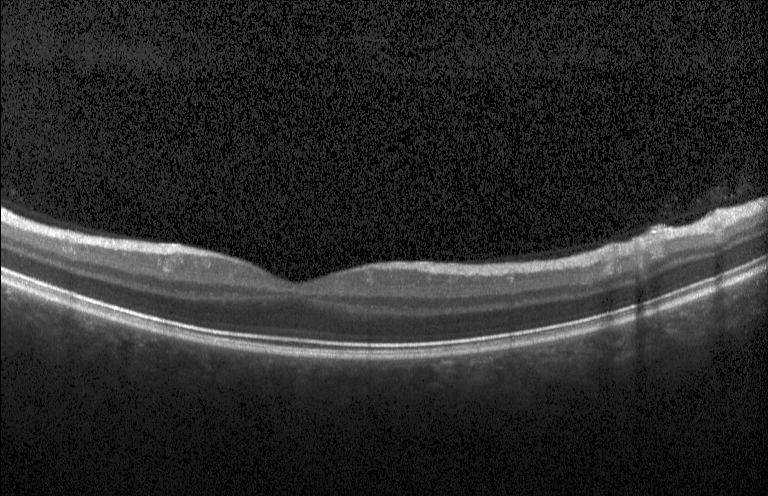 Dx: neither CNV, DME, nor drusen.